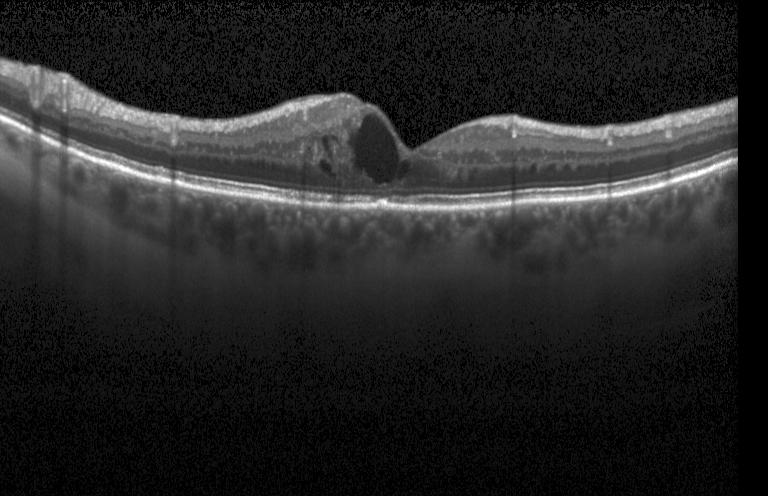 Spectral-domain OCT; retinal OCT cross-section; horizontal scan through the fovea; Heidelberg Spectralis.
Finding: diabetic macular edema.